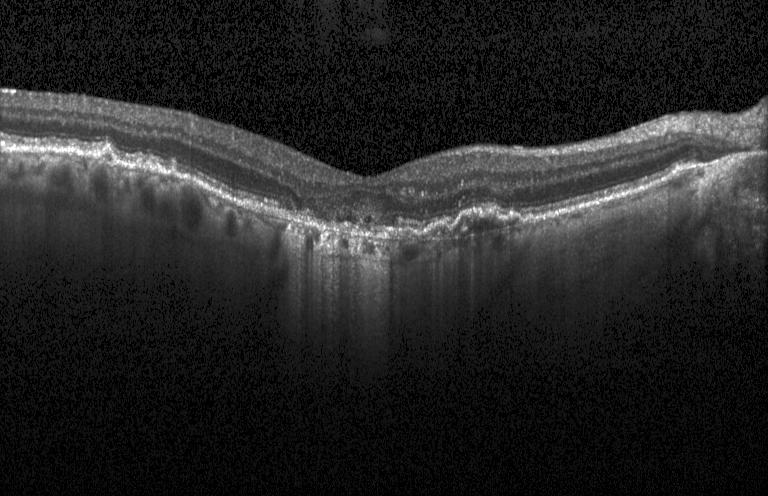
Spectral-domain OCT B-scan: a choroidal neovascular membrane.